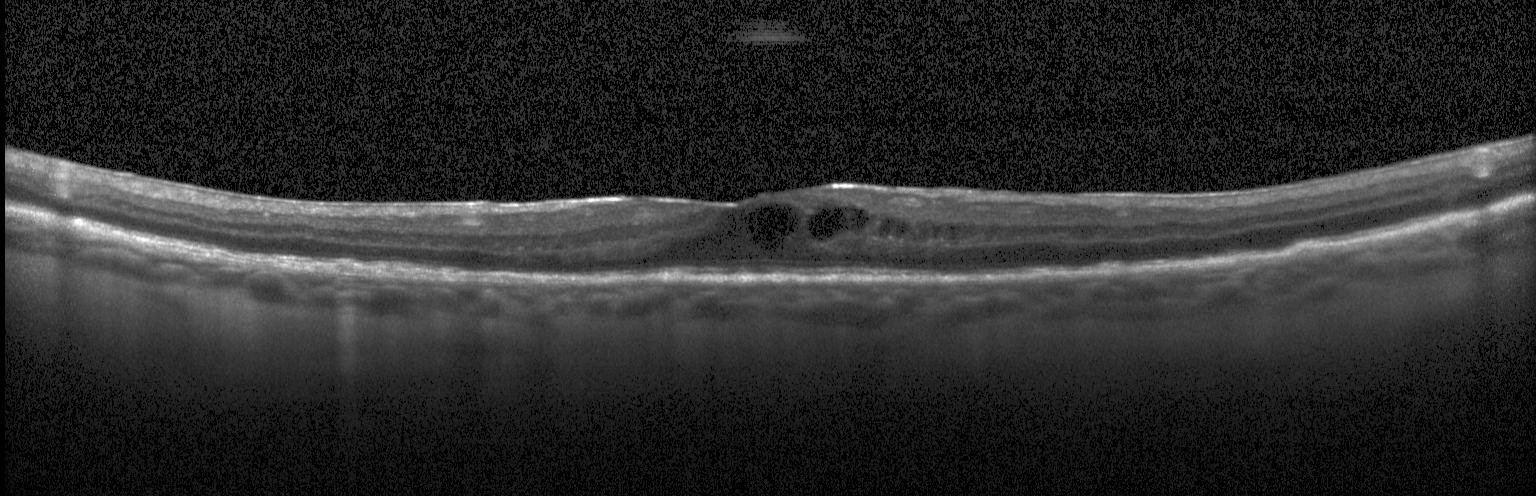 Optical coherence tomography scan — Finding: diabetic macular edema (DME).